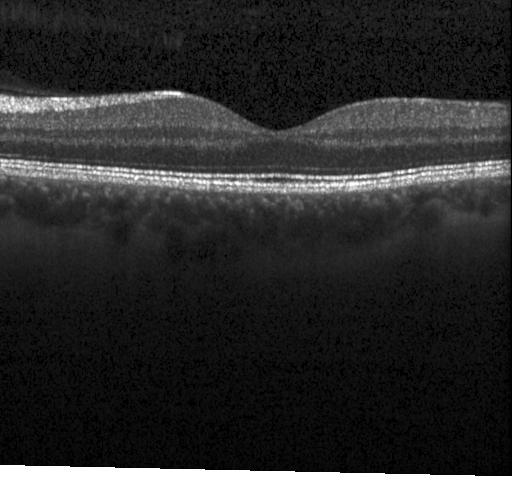

Optical coherence tomography scan.
OCT finding: no evidence of CNV, DME, or drusen.